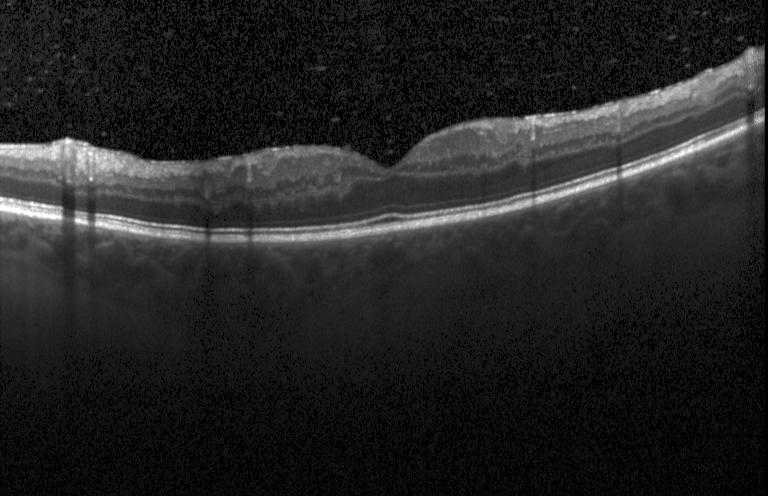
Finding: neither choroidal neovascularization, diabetic macular edema, nor drusen.